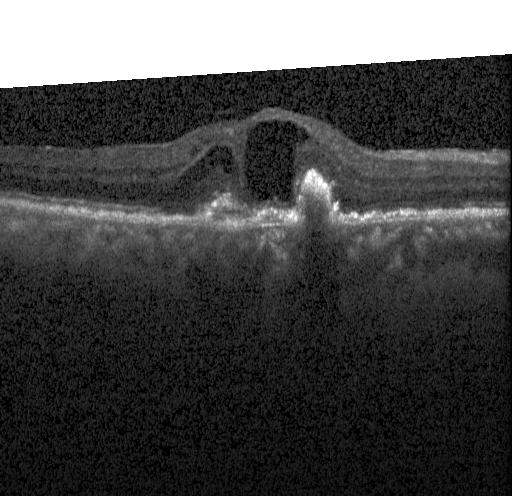

Assessment: CNV.